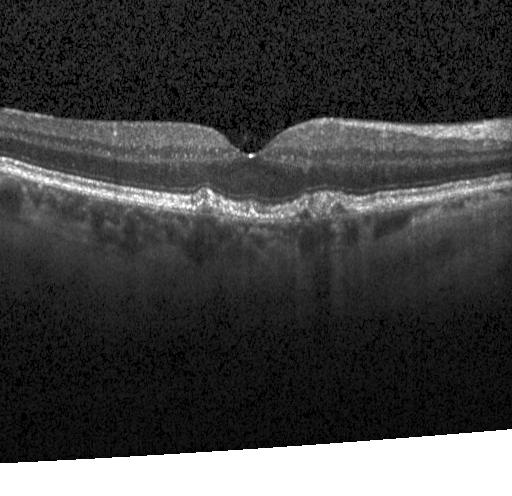
OCT B-scan; macular scan; spectral-domain optical coherence tomography.
Impression: sub-RPE drusenoid deposits.